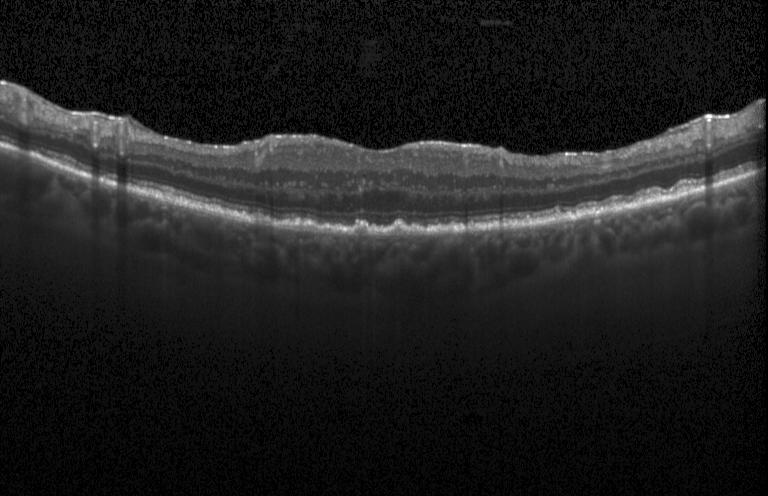

Impression: multiple drusen.